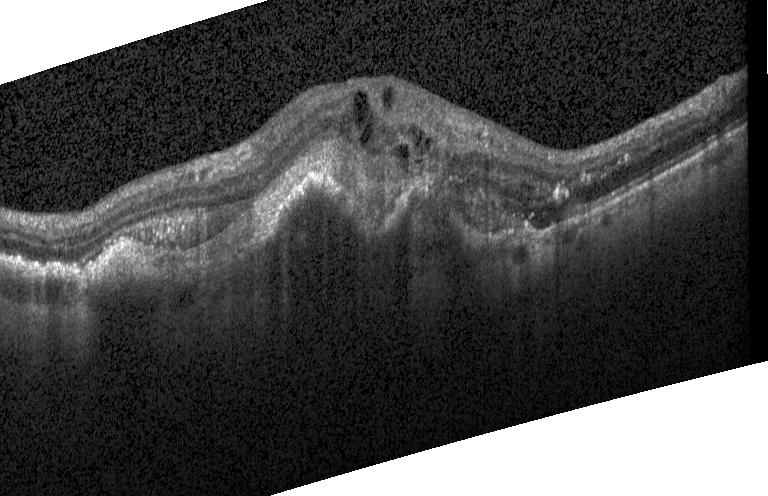
Retinal OCT cross-section.
Assessment: a choroidal neovascular membrane.